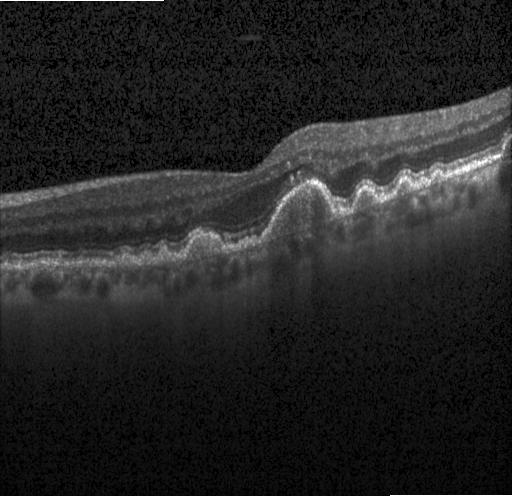 OCT B-scan showing multiple drusen.